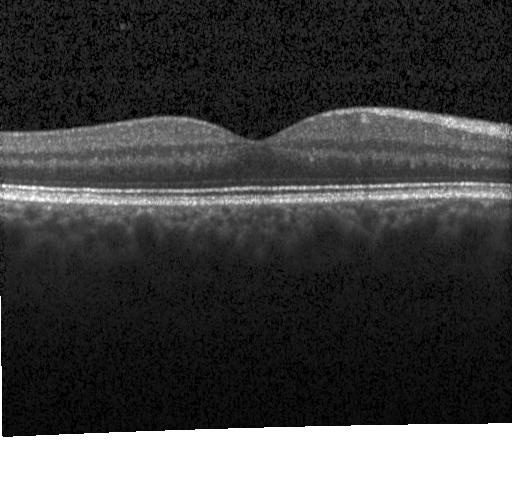 Horizontal scan through the fovea, retinal OCT B-scan. Diagnosis: no CNV, DME, or drusen.